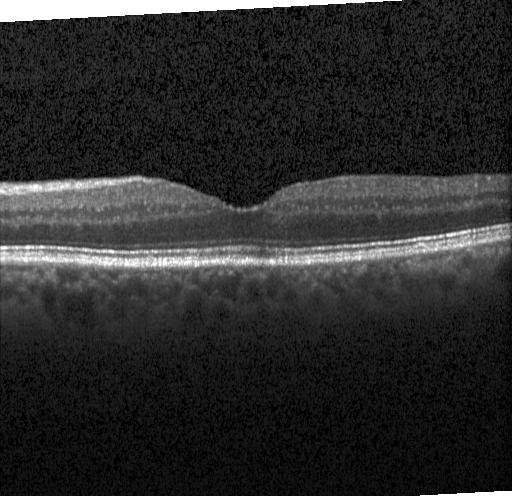
OCT scan showing no evidence of CNV, DME, or drusen.